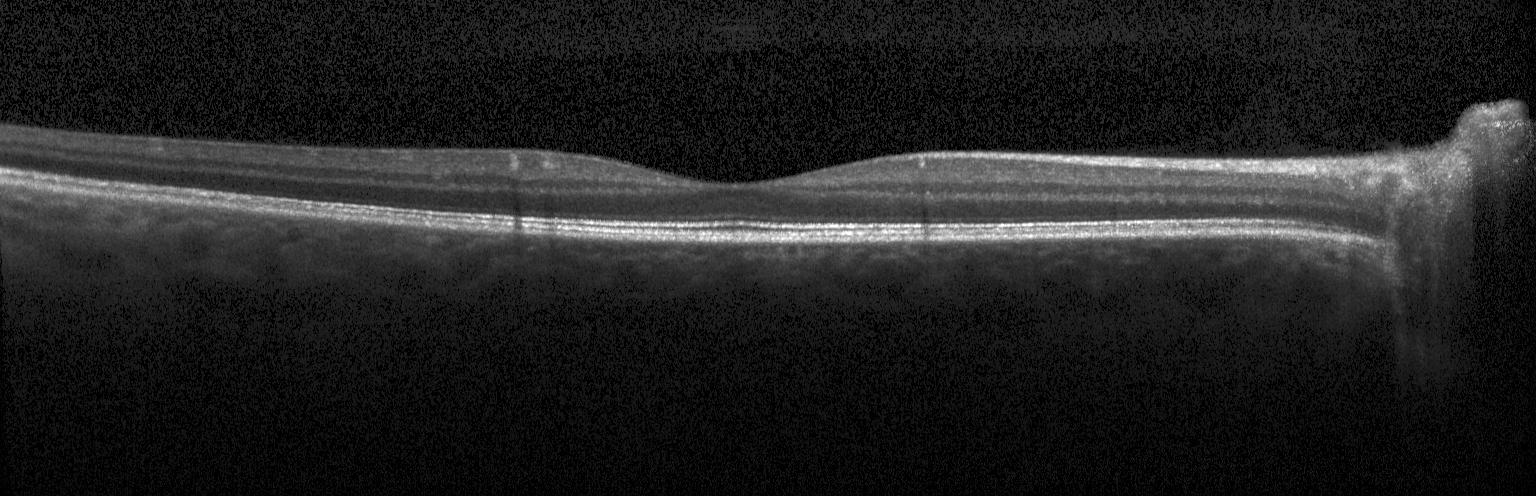
Macular OCT demonstrating neither choroidal neovascularization, diabetic macular edema, nor drusen.